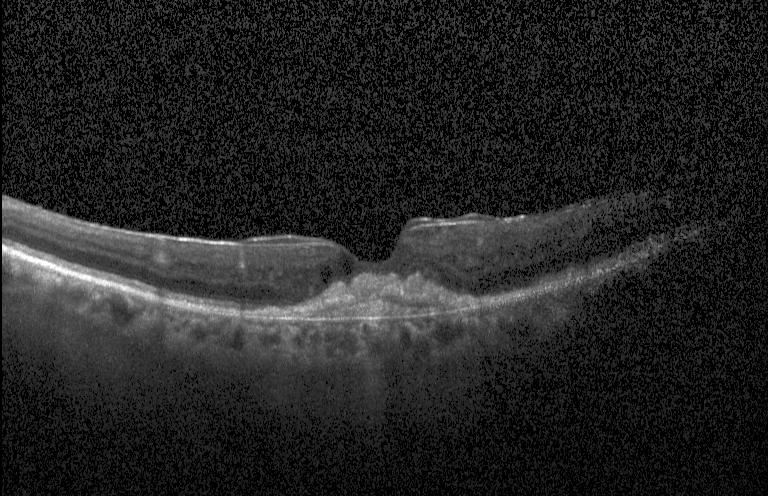

Diagnosis: a choroidal neovascular membrane.